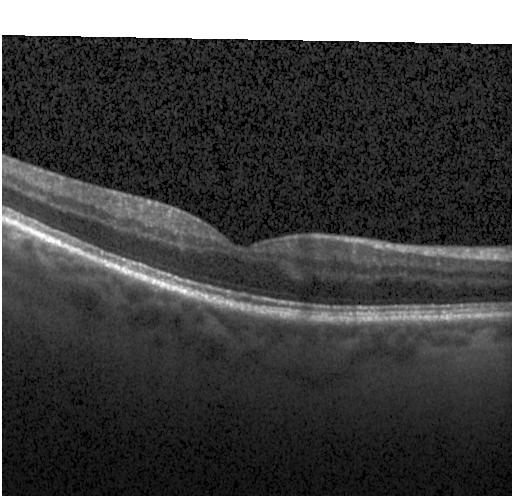

Centered on the fovea. OCT line scan. SD-OCT. Heidelberg Spectralis OCT system
Diagnosis: neither choroidal neovascularization, diabetic macular edema, nor drusen.